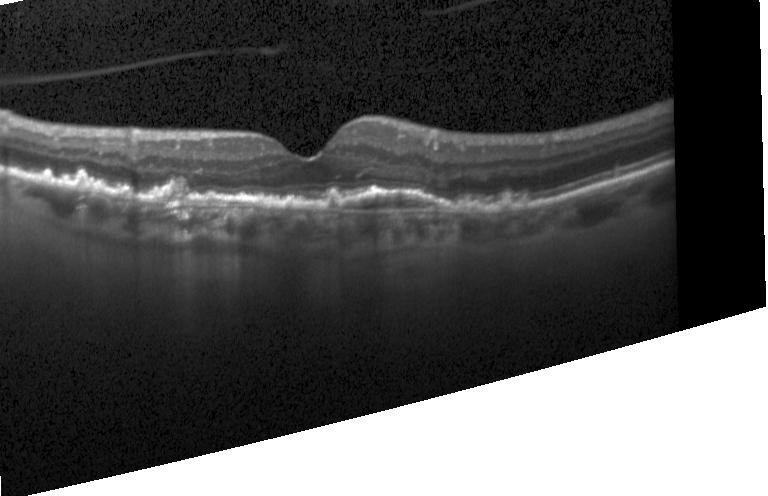
Finding: a choroidal neovascular membrane.